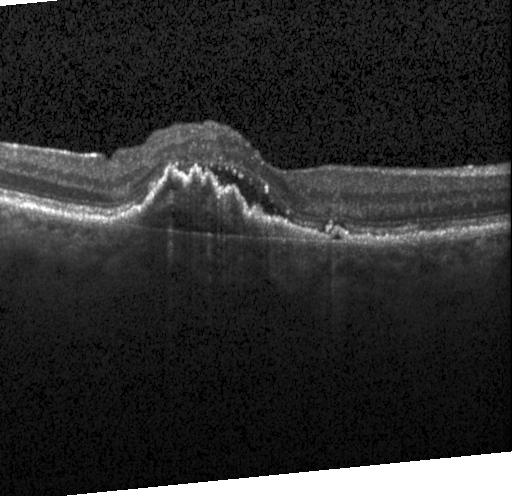
Finding: a choroidal neovascular membrane.